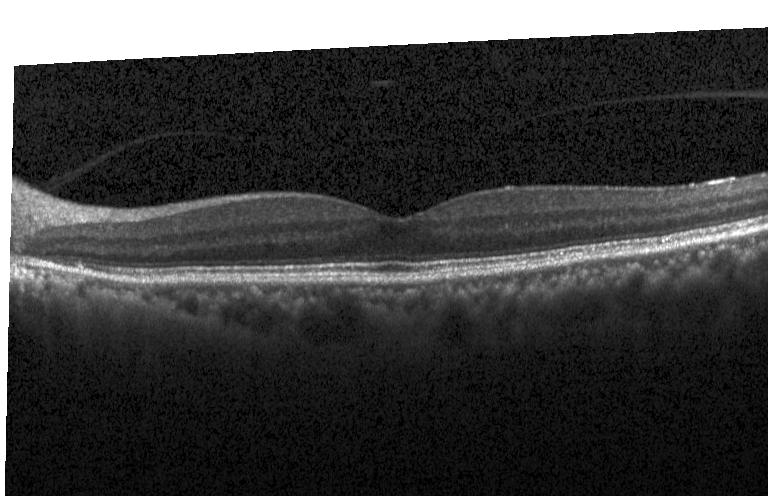 Macular OCT: no choroidal neovascularization, no diabetic macular edema, and no drusen.